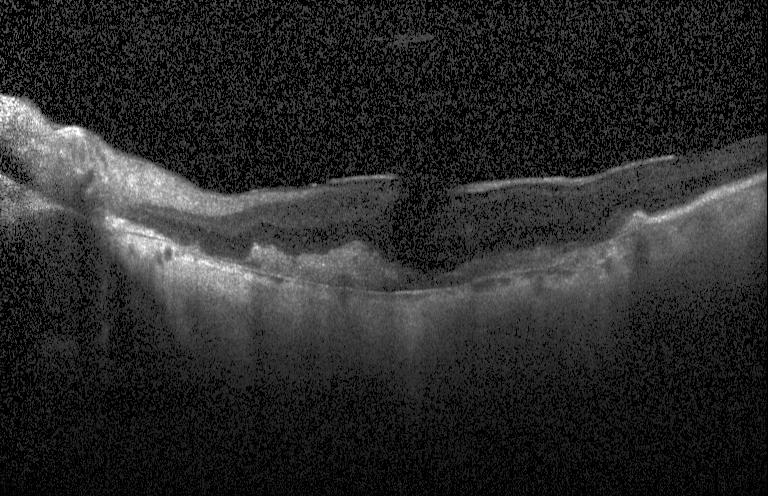

Retinal OCT cross-section
Assessment: choroidal neovascularization.